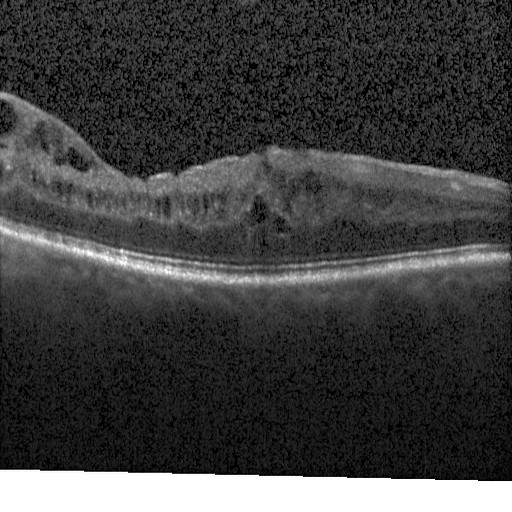
Diagnosis: DME.